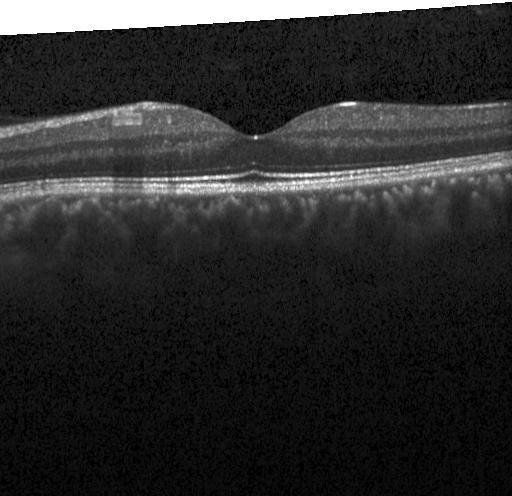
Optical coherence tomography B-scan.
Finding: neither choroidal neovascularization, diabetic macular edema, nor drusen.